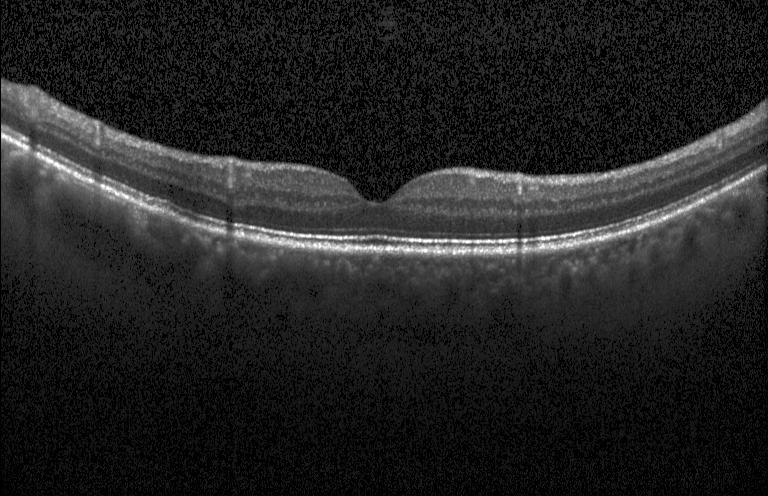

Finding: no CNV, DME, or drusen.